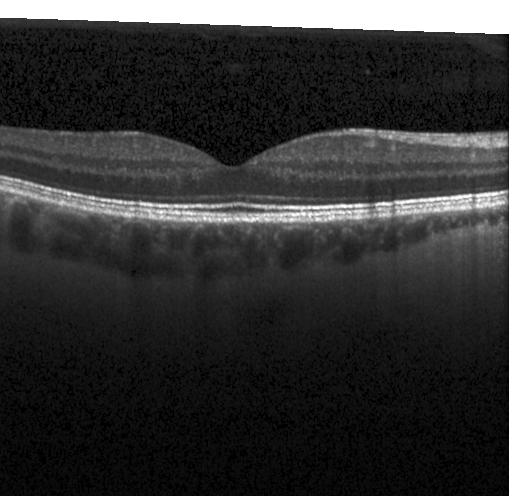
Optical coherence tomography B-scan. Horizontal scan through the fovea. Heidelberg Spectralis OCT system. Spectral-domain optical coherence tomography — Finding: neither choroidal neovascularization, diabetic macular edema, nor drusen.